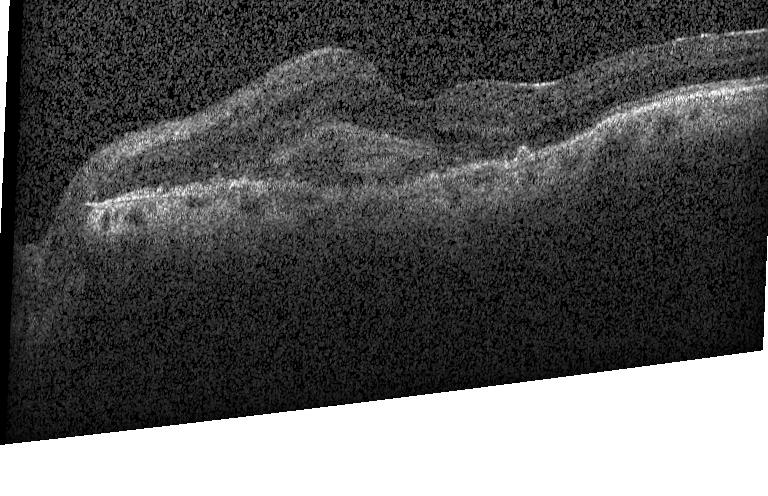 Assessment: CNV.